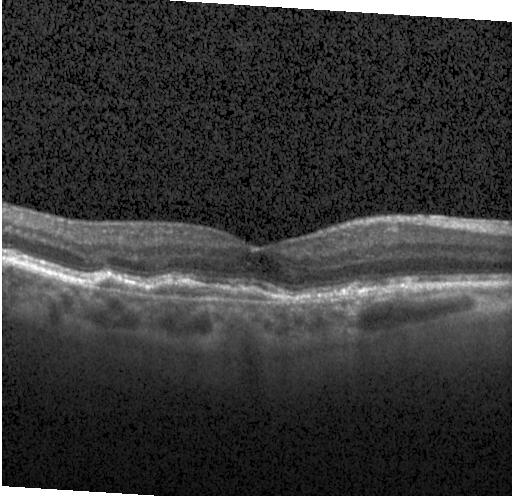 Instrument: Heidelberg Spectralis. Optical coherence tomography scan — Diagnosis: choroidal neovascularization.